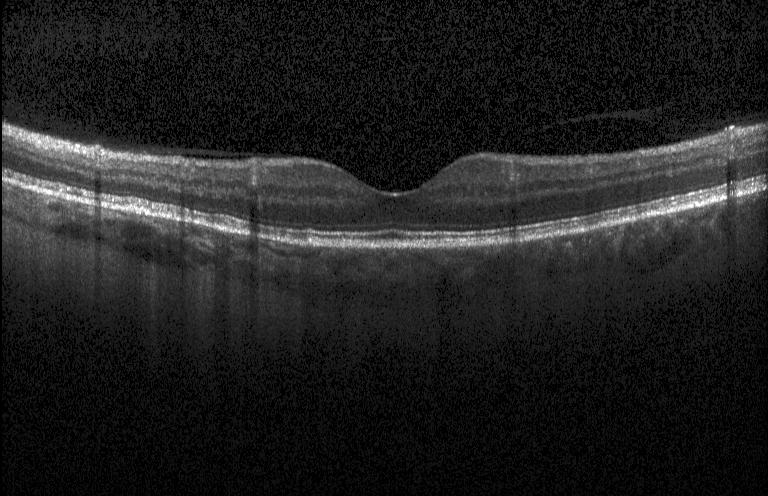
Macular OCT demonstrating neither choroidal neovascularization, diabetic macular edema, nor drusen.